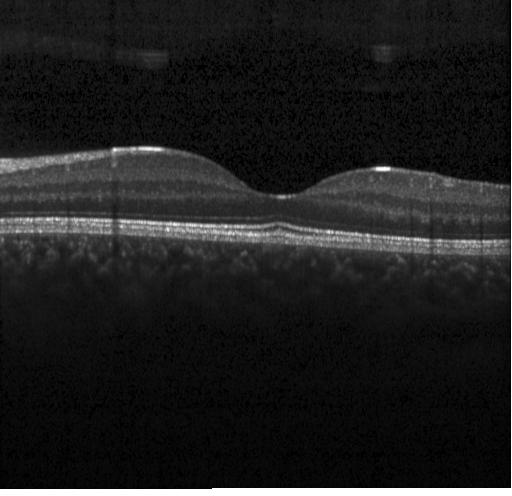 OCT B-scan — Dx: no evidence of choroidal neovascularization, diabetic macular edema, or drusen.